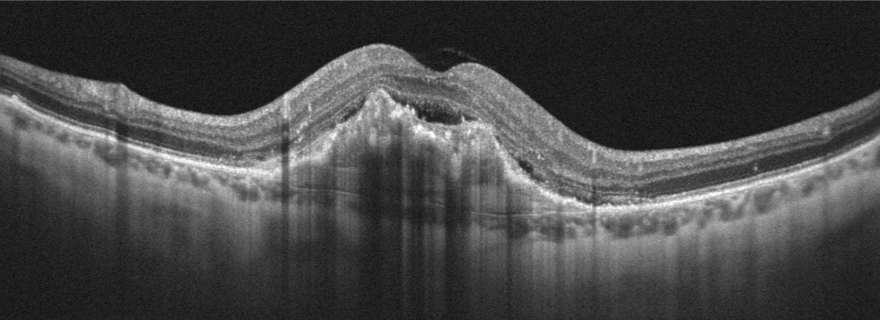
Age-related macular degeneration.